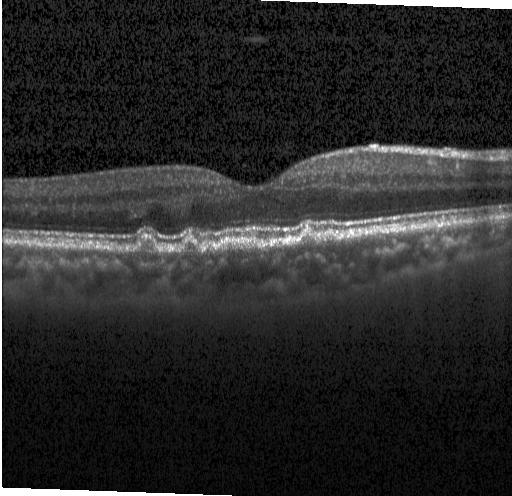 Heidelberg Spectralis OCT system, through the macula, spectral-domain OCT, retinal OCT cross-section.
Impression: sub-RPE drusenoid deposits.